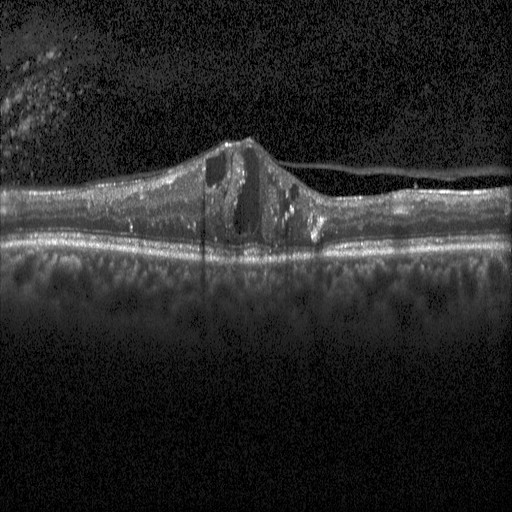

OCT B-scan · Heidelberg Spectralis · macular scan
This B-scan demonstrates diabetic macular edema.